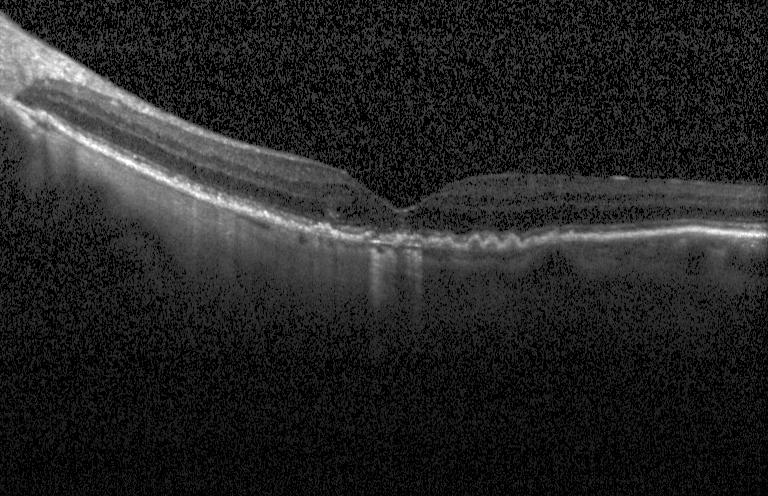 Spectral-domain optical coherence tomography. Acquired on a Heidelberg Spectralis. Retinal OCT cross-section. Horizontal scan through the fovea
This B-scan demonstrates drusen.